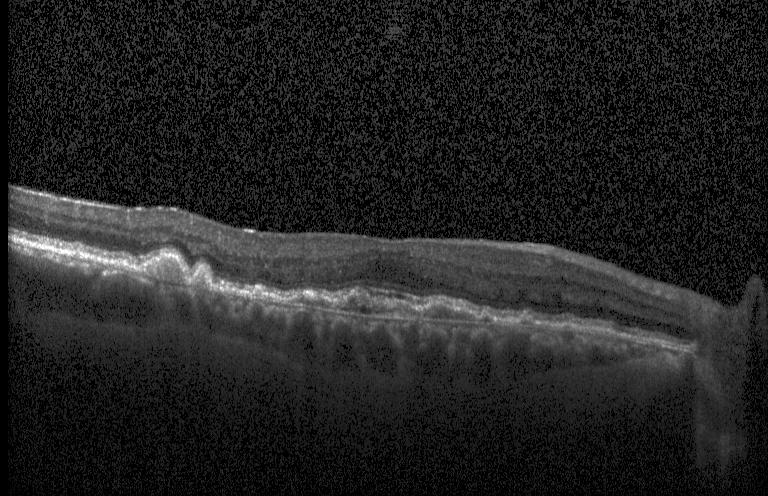
Macular scan, SD-OCT, acquired on a Heidelberg Spectralis, optical coherence tomography scan. Finding: a choroidal neovascular membrane.